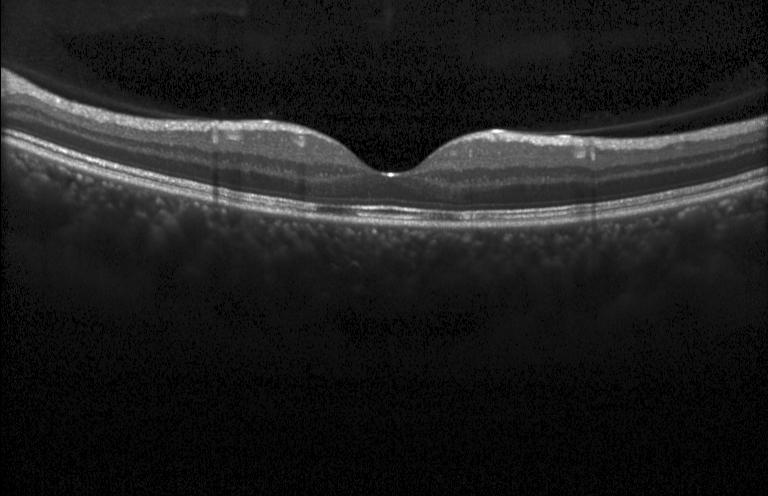

Impression: neither choroidal neovascularization, diabetic macular edema, nor drusen.